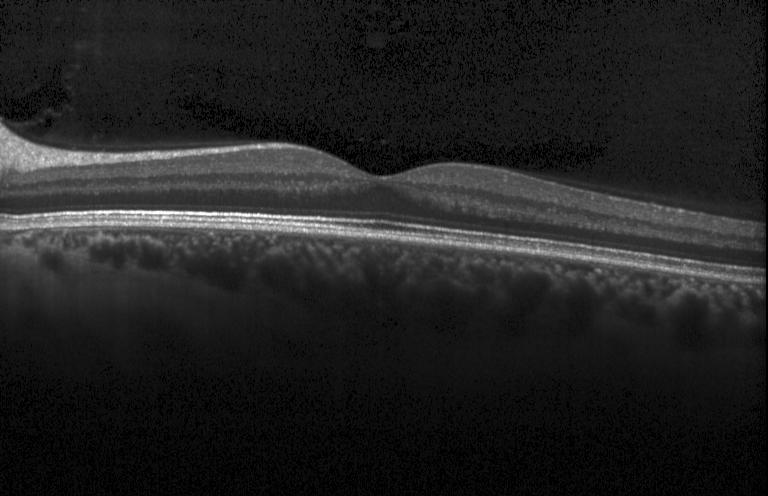
OCT finding: no choroidal neovascularization, diabetic macular edema, or drusen.